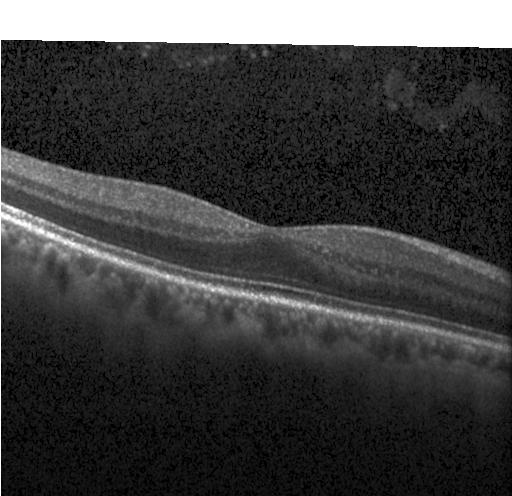
Retinal OCT B-scan.
Diagnosis: no CNV, no DME, and no drusen.